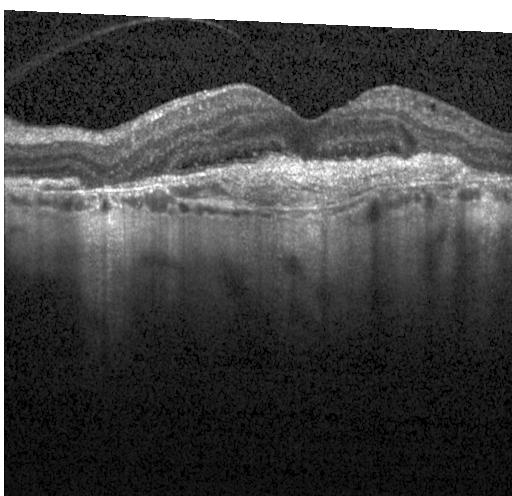

Spectral-domain OCT · optical coherence tomography scan · Heidelberg Spectralis OCT system
Finding: CNV.